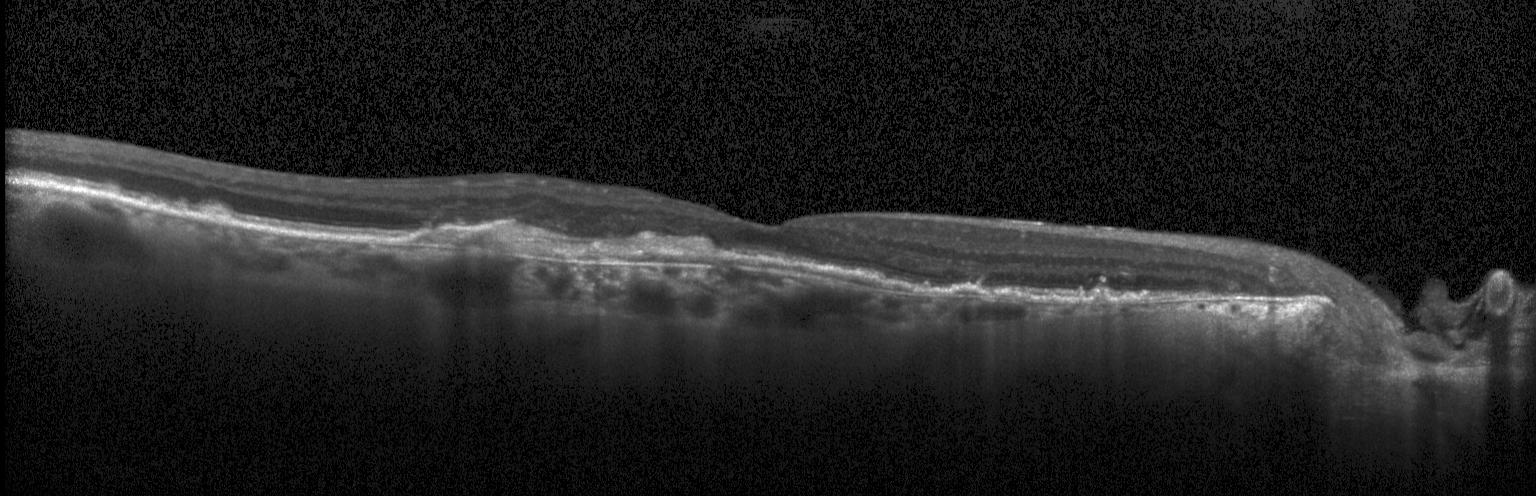

Through the macula, acquired on a Heidelberg Spectralis, OCT line scan, spectral-domain optical coherence tomography.
Diagnosis: a choroidal neovascular membrane.